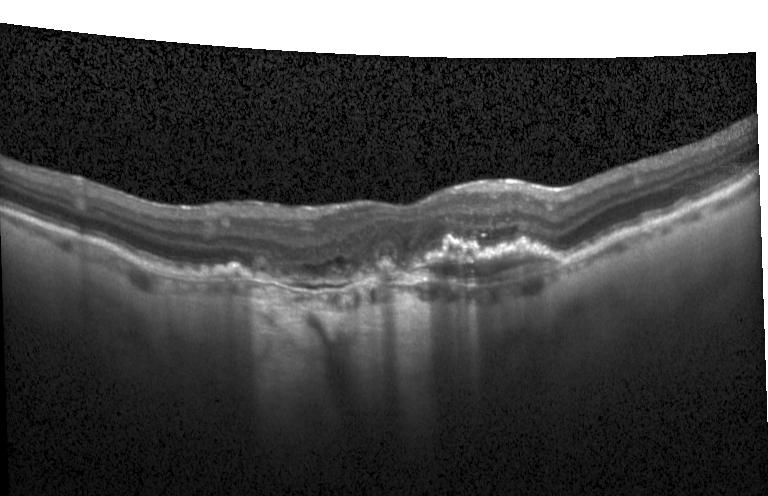 Macular OCT: a choroidal neovascular membrane.